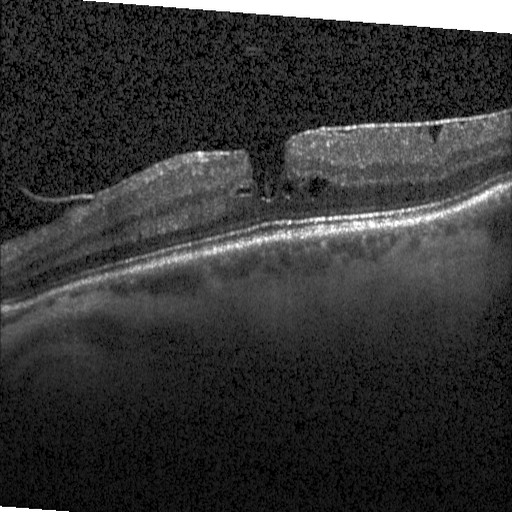 OCT finding: DME.